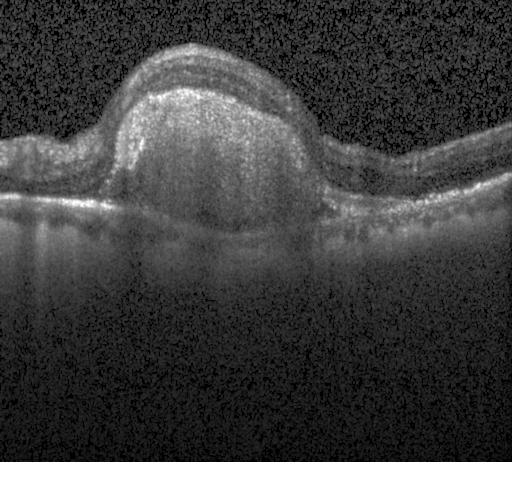

Spectral-domain OCT · acquired on a Heidelberg Spectralis · OCT line scan. Finding: a choroidal neovascular membrane.